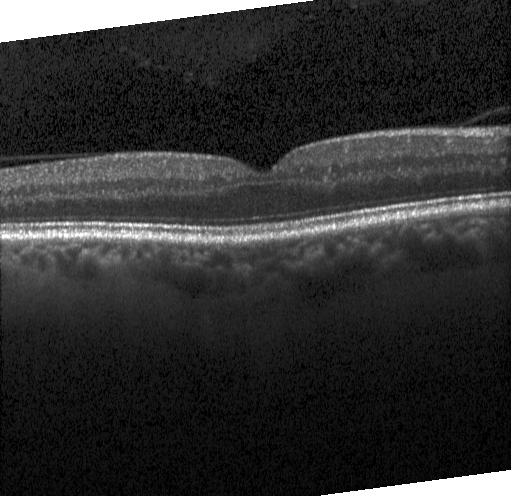 Spectral-domain OCT, acquired on a Heidelberg Spectralis, centered on the fovea, retinal OCT B-scan — Diagnosis: no choroidal neovascularization, diabetic macular edema, or drusen.